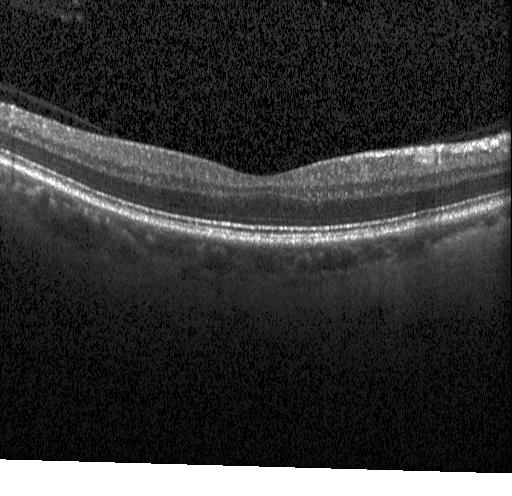
Optical coherence tomography scan. Diagnosis: no choroidal neovascularization, no diabetic macular edema, and no drusen.